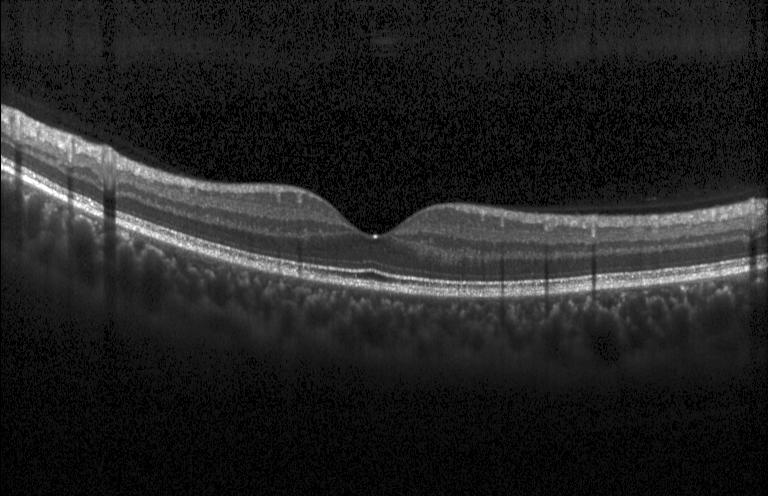 Through the macula. Optical coherence tomography scan. Finding: no evidence of choroidal neovascularization, diabetic macular edema, or drusen.